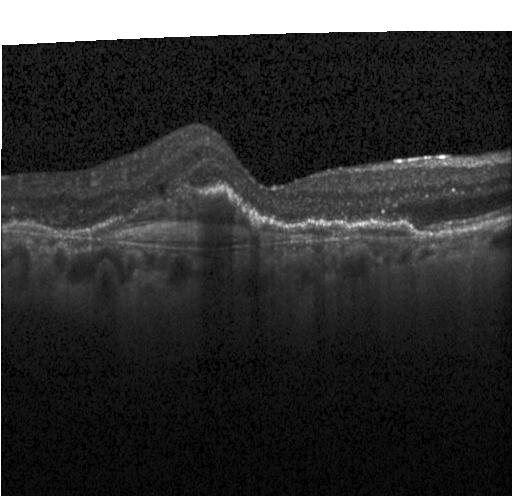
Horizontal scan through the fovea; optical coherence tomography scan; acquired on a Heidelberg Spectralis; spectral-domain optical coherence tomography.
This B-scan demonstrates a choroidal neovascular membrane.